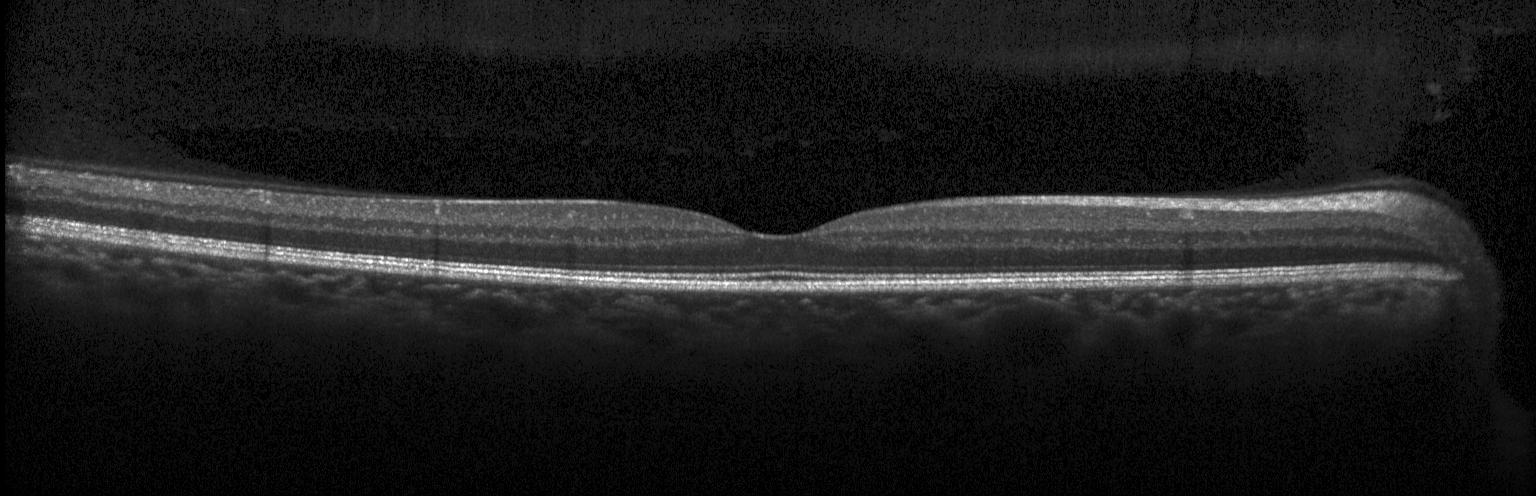 Optical coherence tomography B-scan. Finding: no choroidal neovascularization, diabetic macular edema, or drusen.